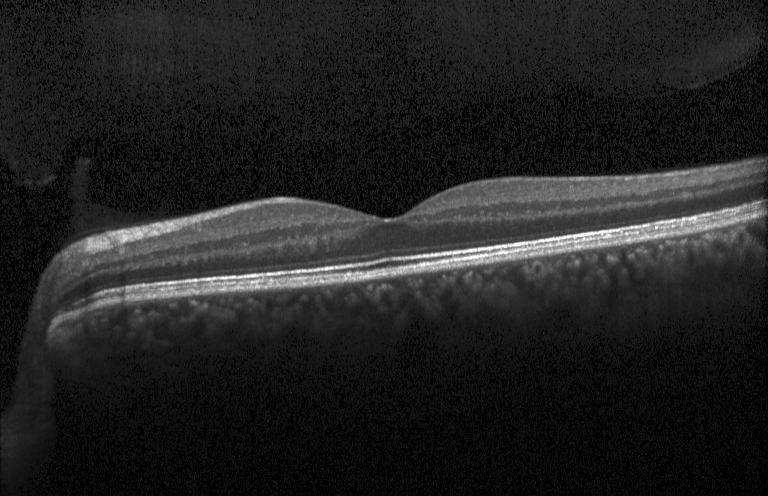
Acquired on a Heidelberg Spectralis, spectral-domain OCT, macular scan, OCT line scan.
Impression: no evidence of choroidal neovascularization, diabetic macular edema, or drusen.